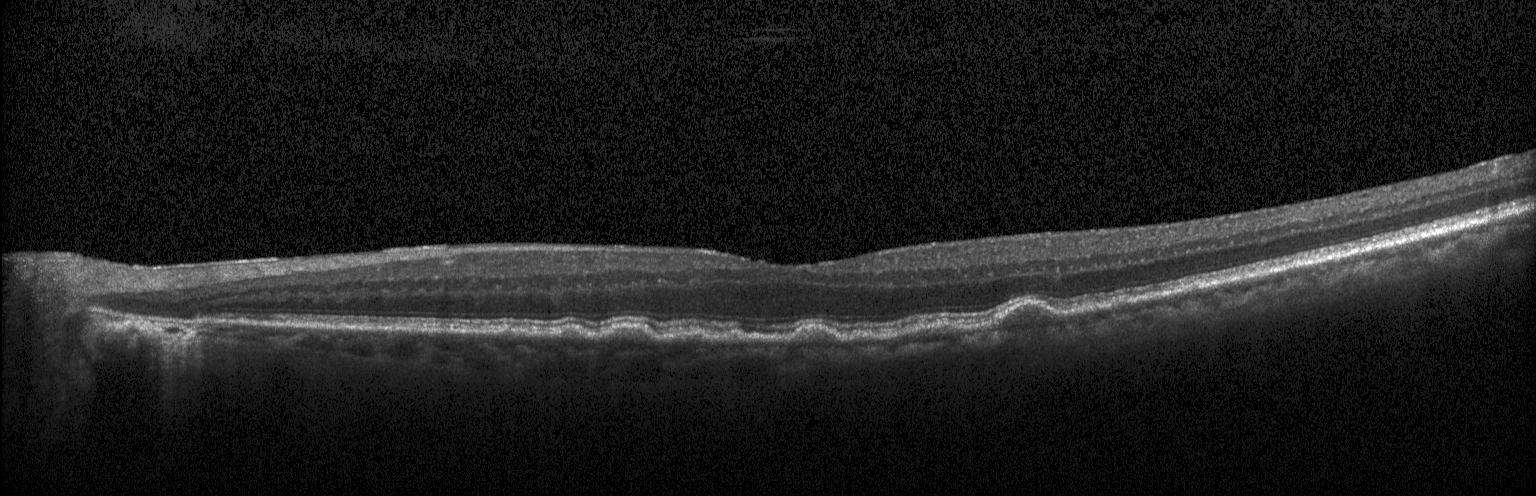
Heidelberg Spectralis OCT system. Retinal OCT cross-section.
Impression: sub-RPE drusenoid deposits.